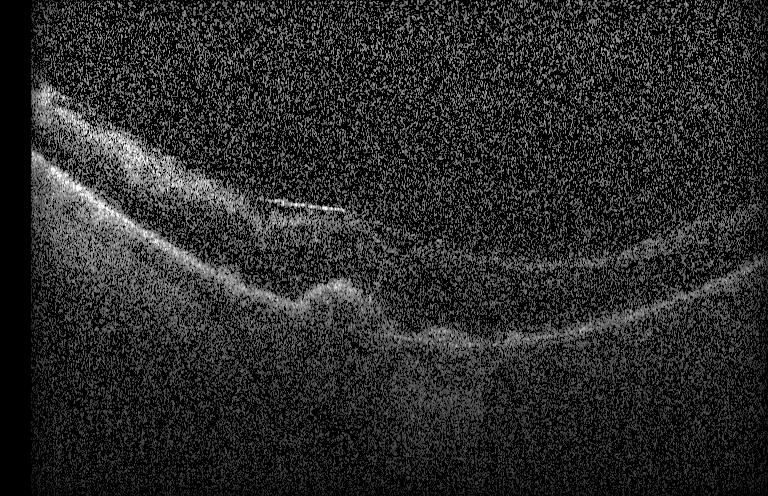
Centered on the fovea, SD-OCT, optical coherence tomography scan, instrument: Heidelberg Spectralis
This B-scan demonstrates choroidal neovascularization (CNV).